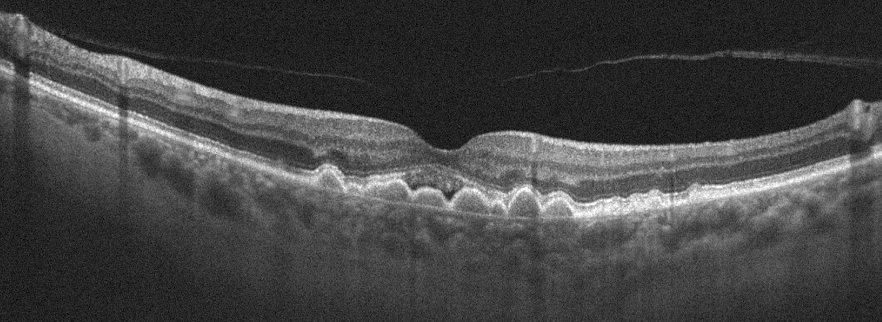
OCT line scan. Diagnosis: age-related macular degeneration (AMD).